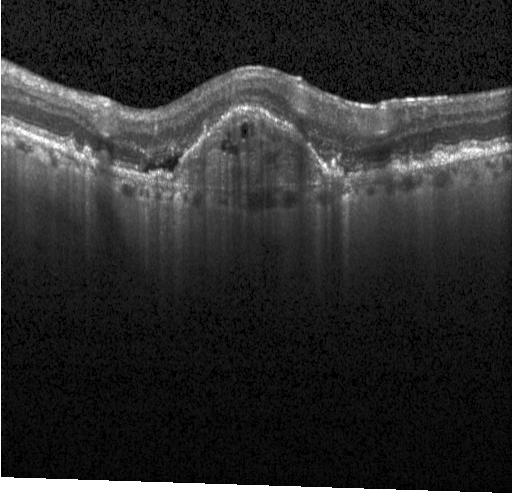 OCT line scan; acquired on a Heidelberg Spectralis
Impression: choroidal neovascularization.